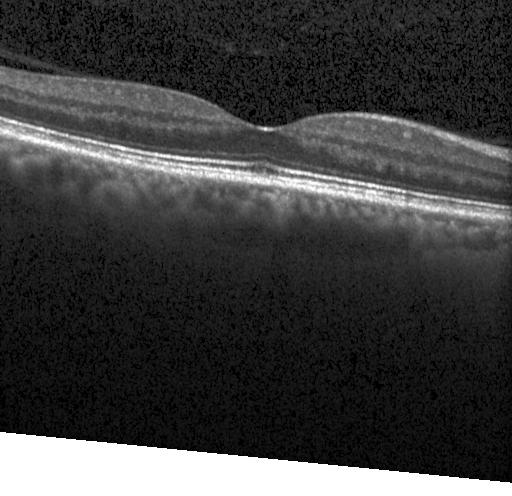 Diagnosis: no evidence of choroidal neovascularization, diabetic macular edema, or drusen.